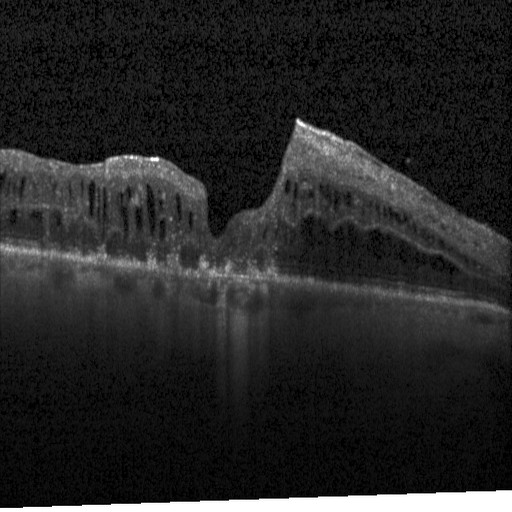
Finding: diabetic macular edema (DME).